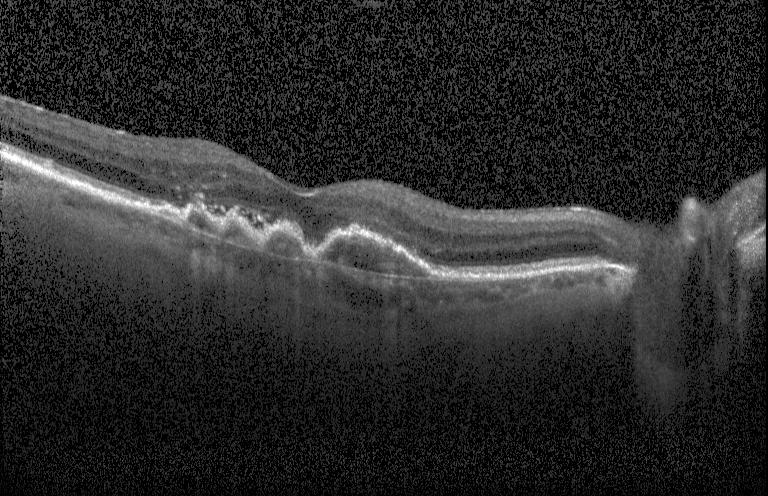 Diagnosis: a choroidal neovascular membrane.